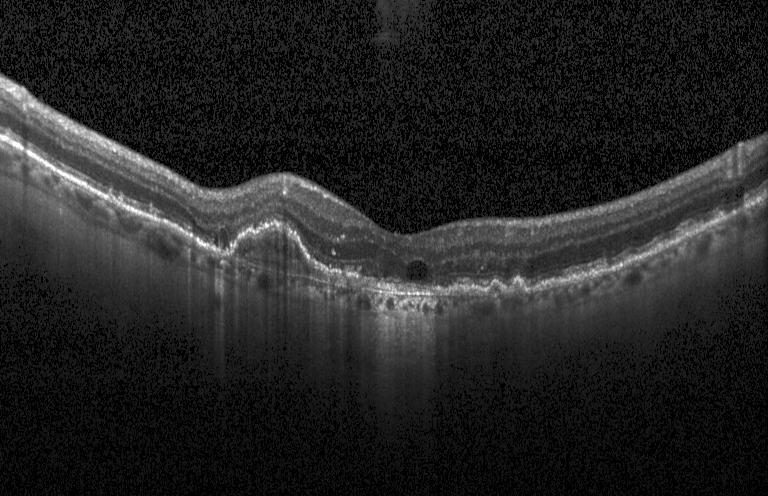 Dx: choroidal neovascularization (CNV).